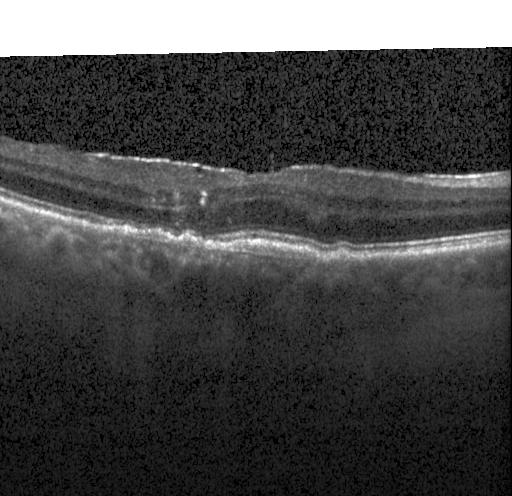

OCT line scan; instrument: Heidelberg Spectralis; fovea-centered; SD-OCT — This B-scan demonstrates a choroidal neovascular membrane.